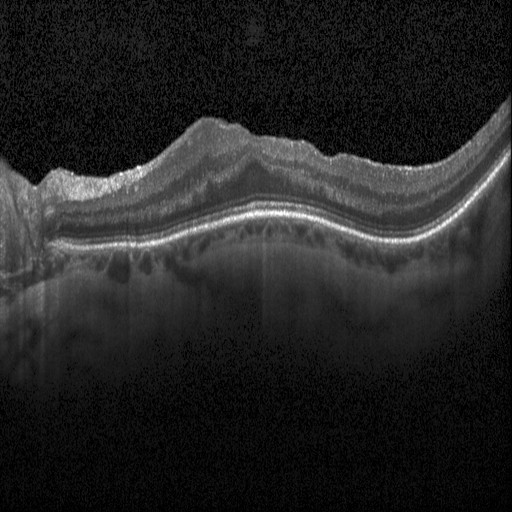 Optical coherence tomography scan · instrument: Heidelberg Spectralis.
This B-scan demonstrates diabetic macular edema (DME).